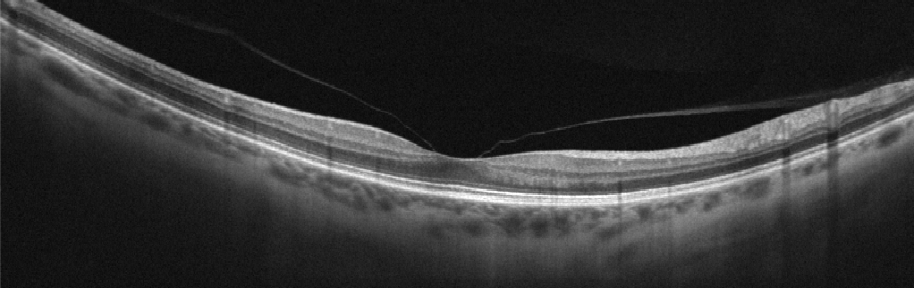
Optical coherence tomography scan
This B-scan demonstrates no AMD, DME, ERM, RAO, RVO, or VID.